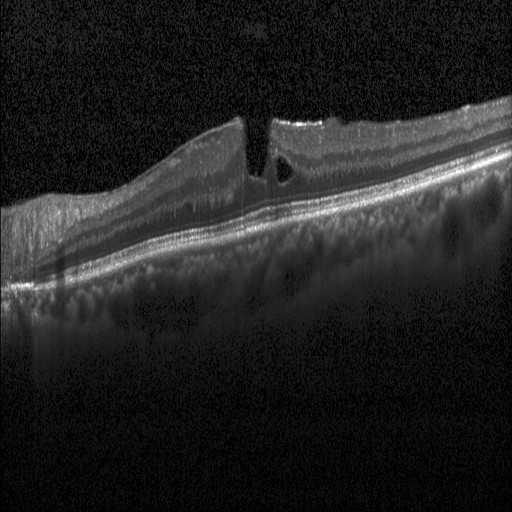

Impression: diabetic macular edema (DME).